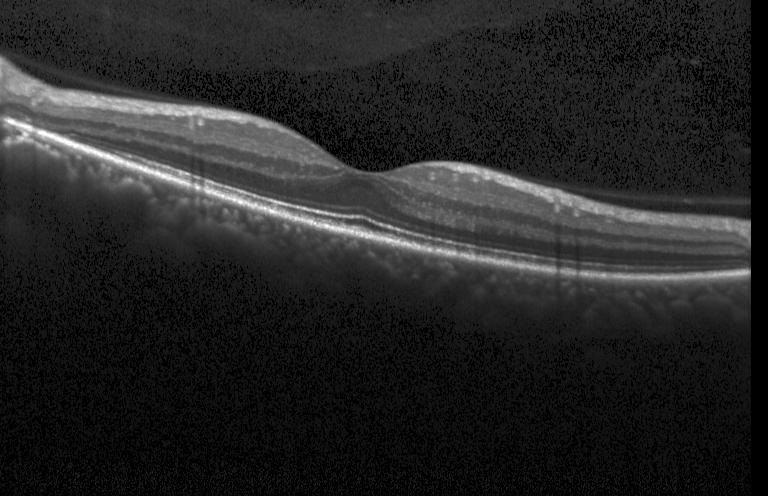

OCT line scan, SD-OCT — Finding: neither choroidal neovascularization, diabetic macular edema, nor drusen.